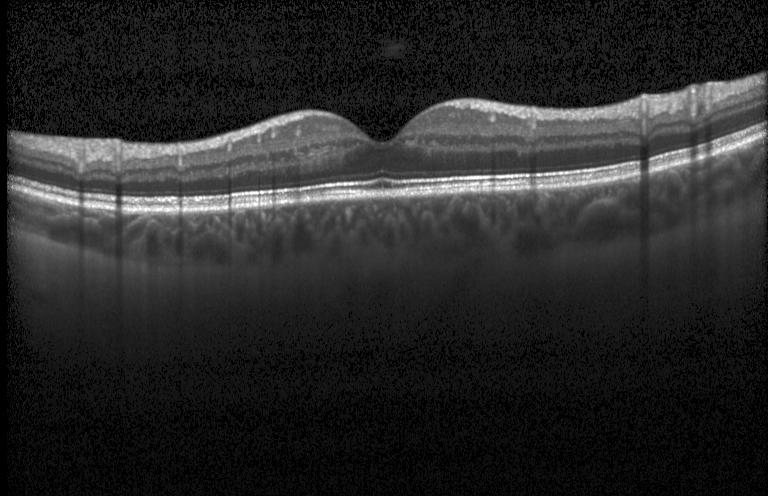 Dx: no evidence of choroidal neovascularization, diabetic macular edema, or drusen.